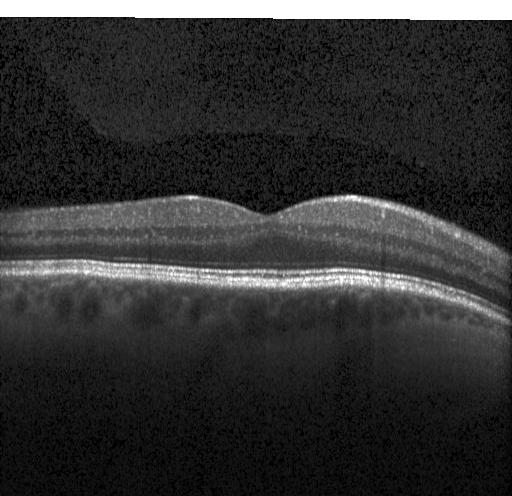 Impression: no choroidal neovascularization, diabetic macular edema, or drusen.